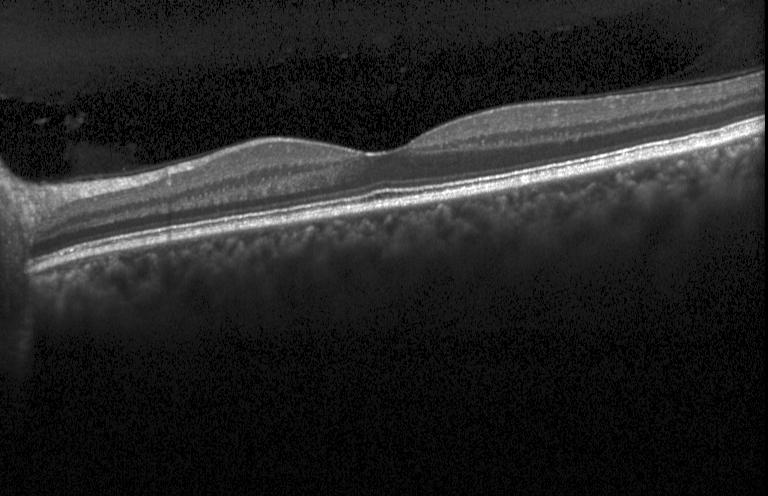
Retinal OCT cross-section · spectral-domain optical coherence tomography · instrument: Heidelberg Spectralis · through the macula.
OCT finding: neither CNV, DME, nor drusen.